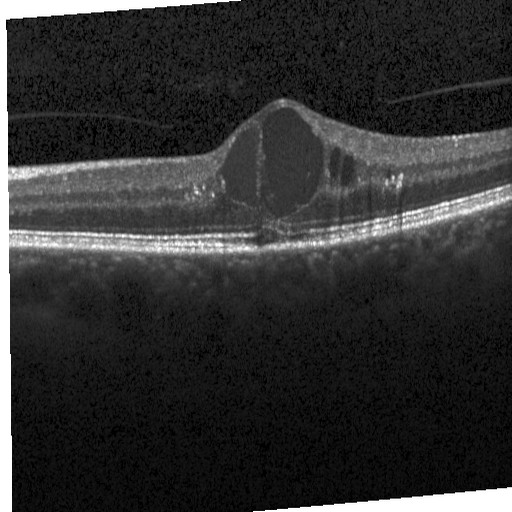 Retinal OCT B-scan, centered on the fovea, SD-OCT. Macular OCT: DME.